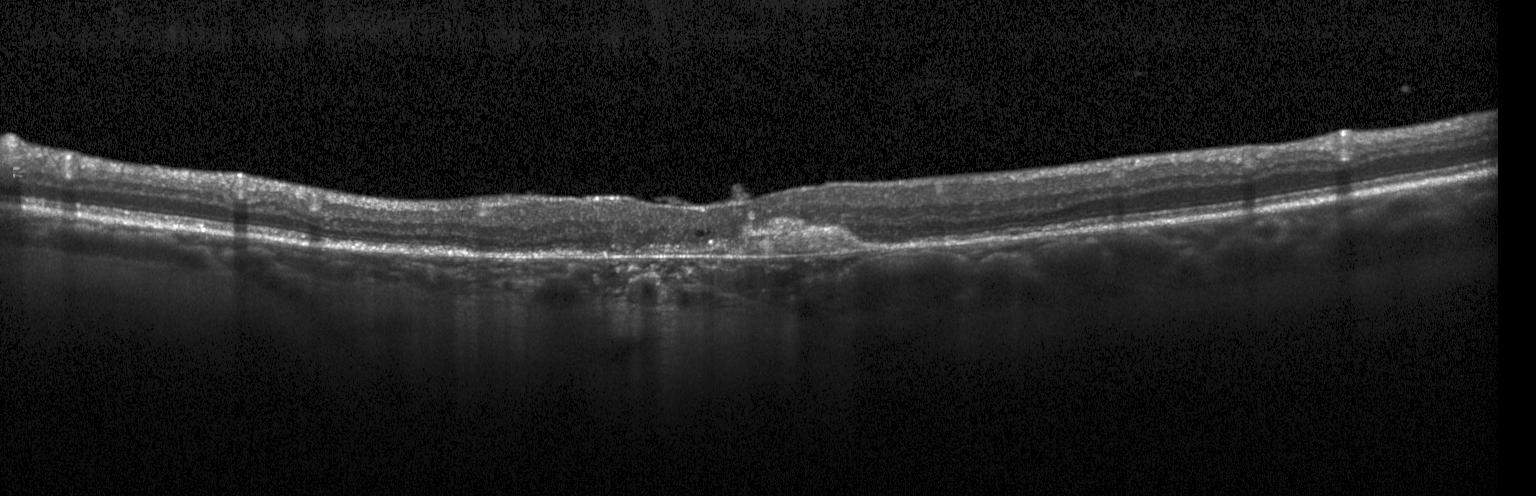

OCT line scan · spectral-domain OCT.
Dx: a choroidal neovascular membrane.